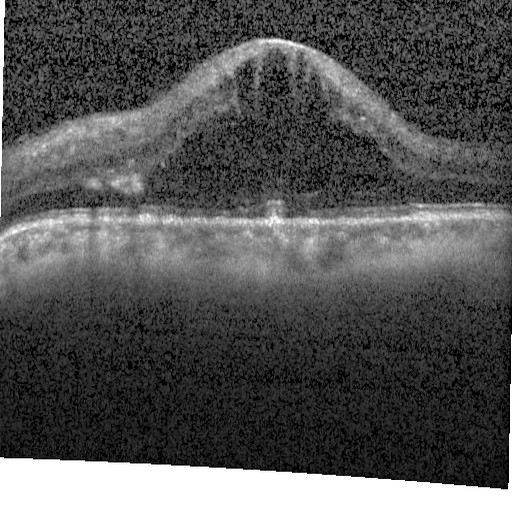 Heidelberg Spectralis. OCT B-scan. Centered on the fovea.
Impression: diabetic macular edema (DME).